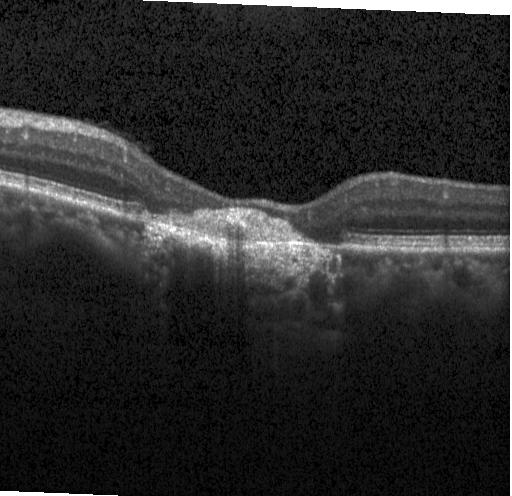

OCT line scan.
Impression: a choroidal neovascular membrane.